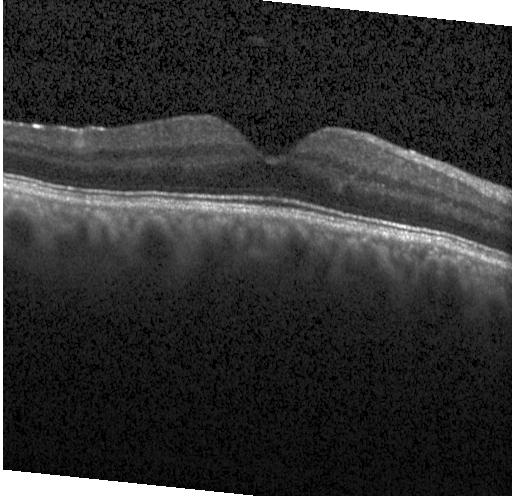
Optical coherence tomography B-scan, spectral-domain optical coherence tomography — OCT finding: no choroidal neovascularization, no diabetic macular edema, and no drusen.